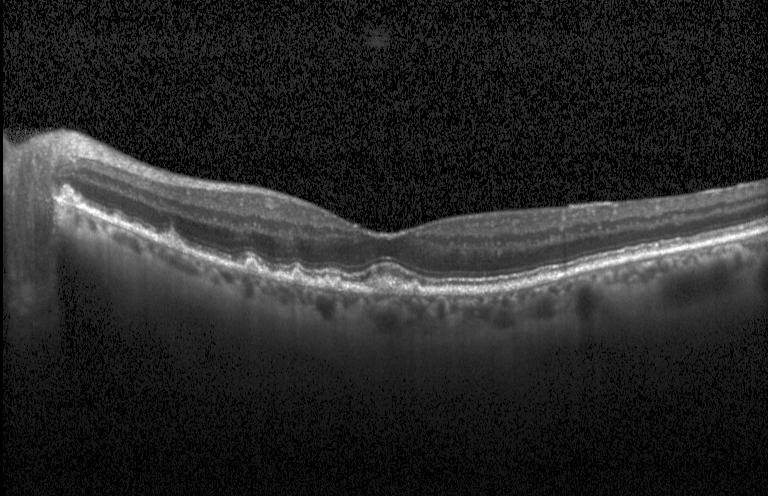 Optical coherence tomography scan. Instrument: Heidelberg Spectralis. SD-OCT. Drusen.